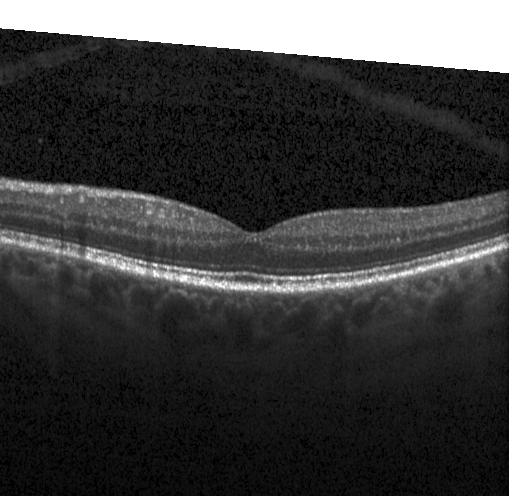 Spectral-domain optical coherence tomography. Horizontal scan through the fovea. Heidelberg Spectralis. Optical coherence tomography B-scan.
Macular OCT: no choroidal neovascularization, no diabetic macular edema, and no drusen.